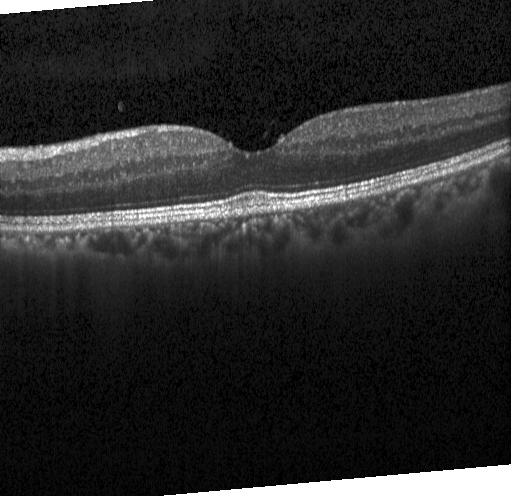

Diagnosis: no evidence of choroidal neovascularization, diabetic macular edema, or drusen.